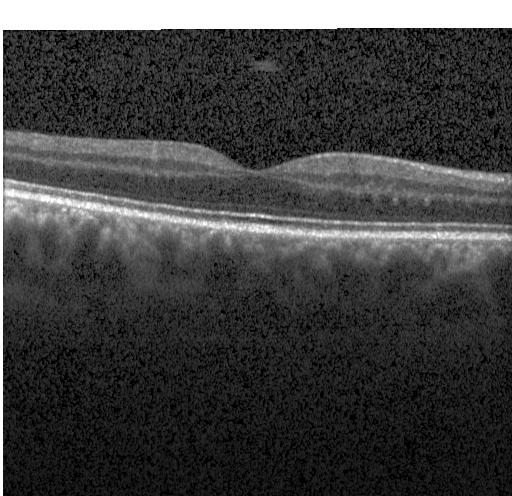 Retinal OCT cross-section · through the macula · spectral-domain OCT — Dx: no choroidal neovascularization, diabetic macular edema, or drusen.